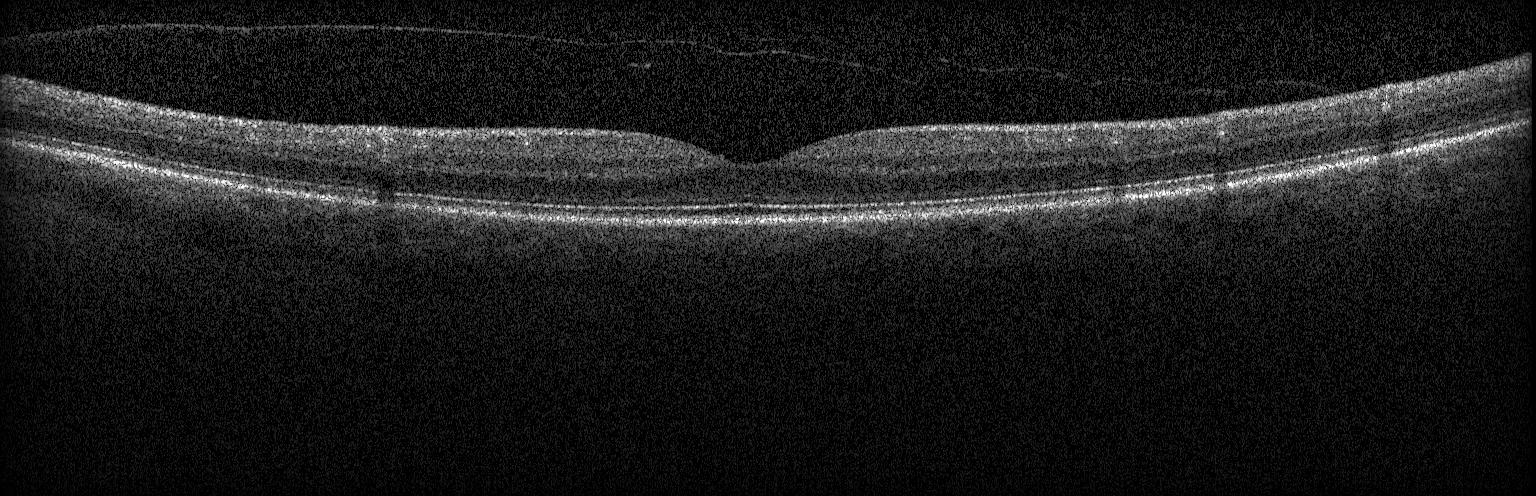
Optical coherence tomography B-scan
Macular OCT: no CNV, no DME, and no drusen.